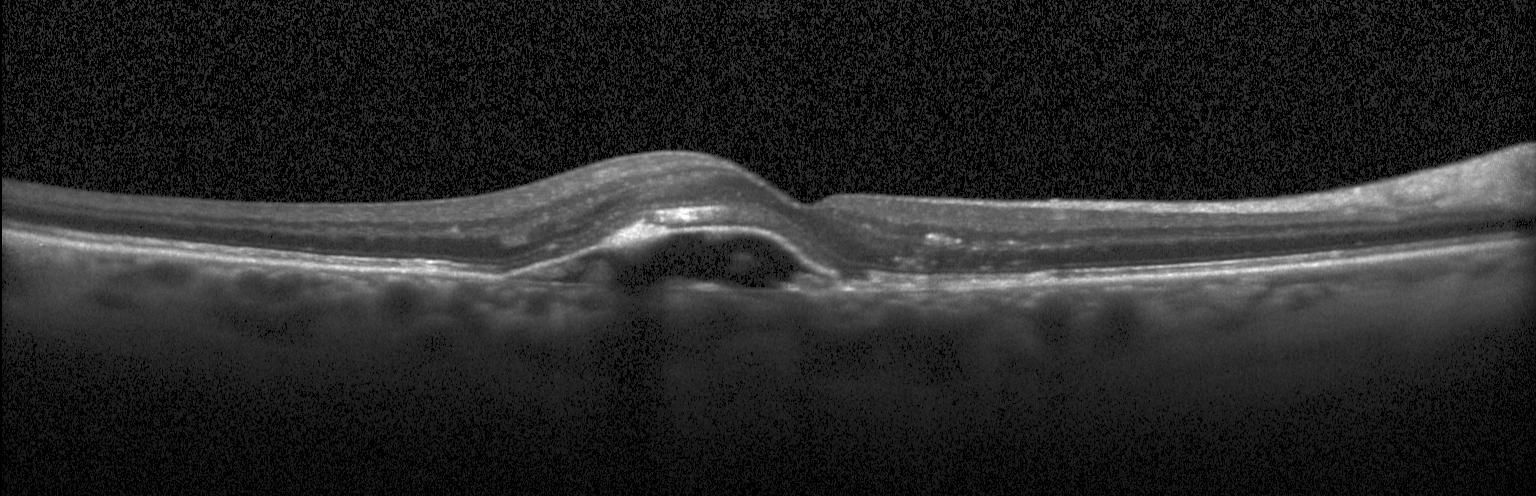

OCT B-scan · SD-OCT. Assessment: a choroidal neovascular membrane.